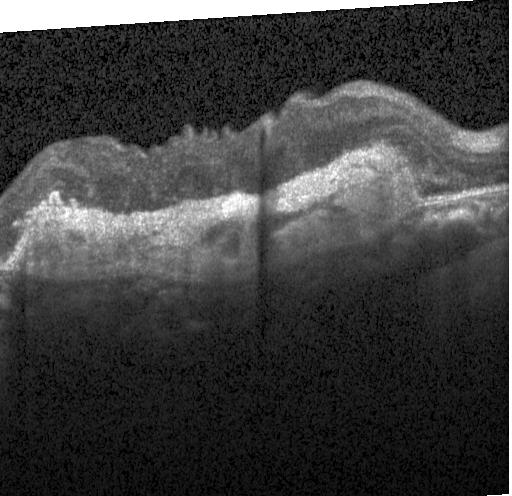
OCT line scan. Dx: choroidal neovascularization.